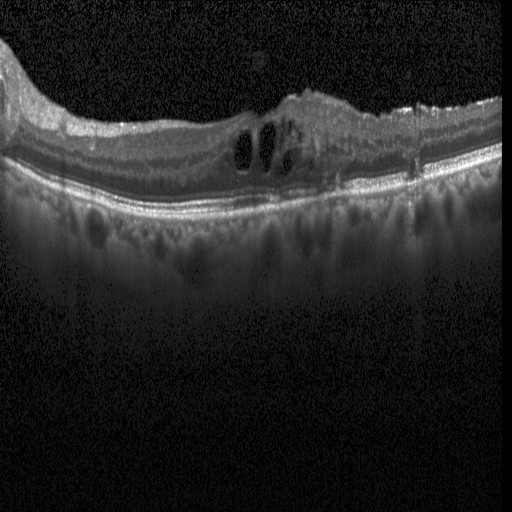

OCT line scan. Finding: diabetic macular edema (DME).